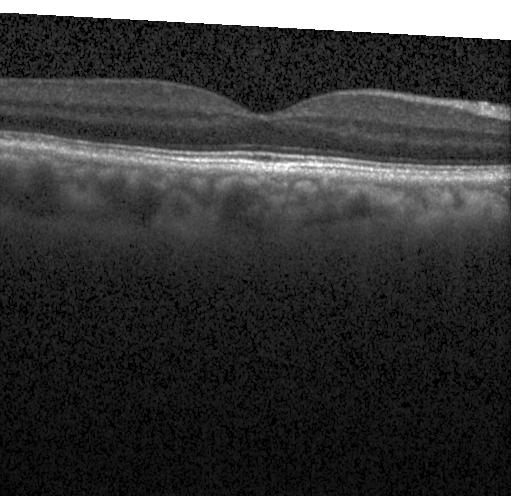

OCT B-scan · Heidelberg Spectralis · fovea-centered.
Diagnosis: no evidence of choroidal neovascularization, diabetic macular edema, or drusen.